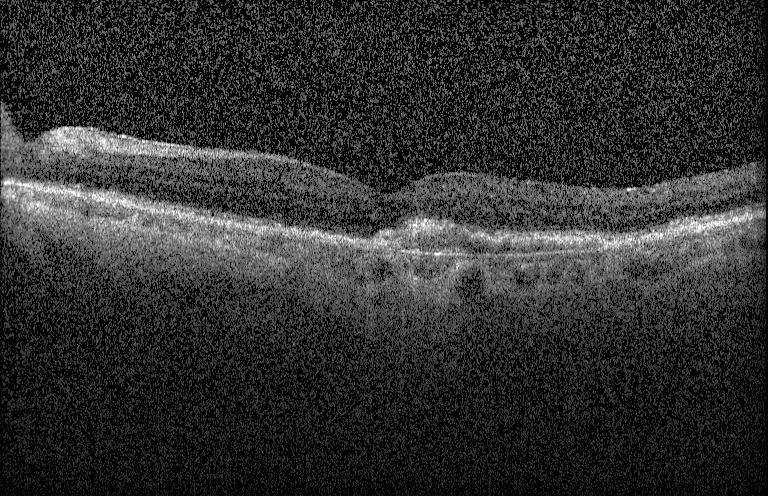
Diagnosis: CNV.